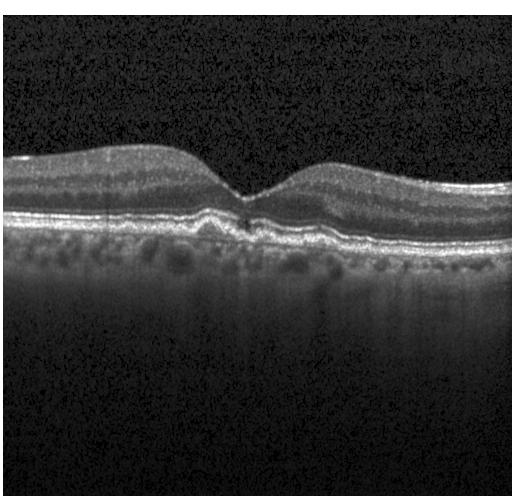

Macular scan · instrument: Heidelberg Spectralis · optical coherence tomography B-scan · SD-OCT — Finding: sub-RPE drusenoid deposits.